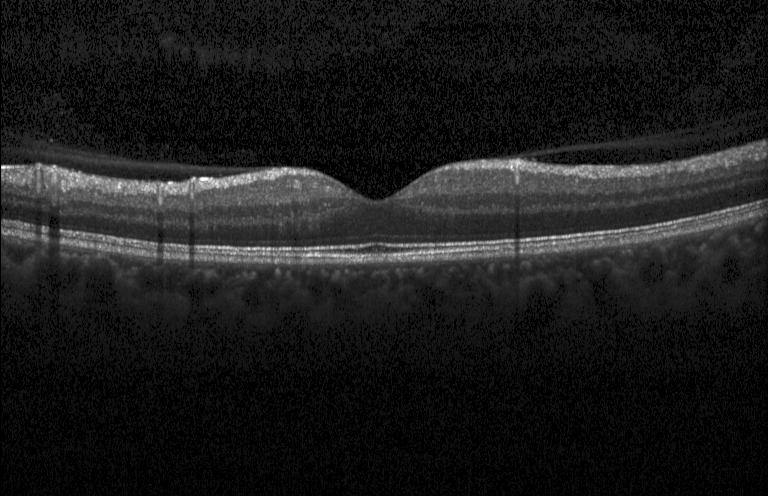

OCT B-scan. SD-OCT — This B-scan demonstrates no choroidal neovascularization, diabetic macular edema, or drusen.